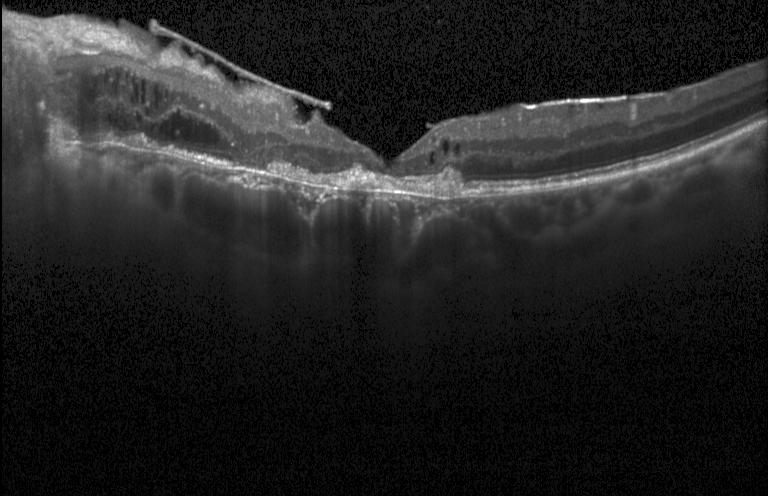 Diagnosis: a choroidal neovascular membrane.